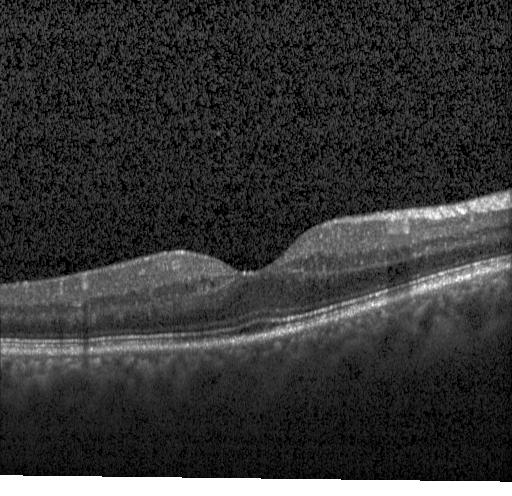 Retinal OCT B-scan. Impression: neither choroidal neovascularization, diabetic macular edema, nor drusen.